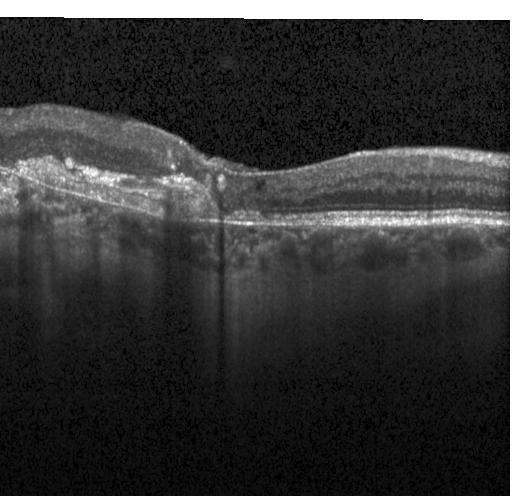 OCT B-scan, instrument: Heidelberg Spectralis. Impression: a choroidal neovascular membrane.